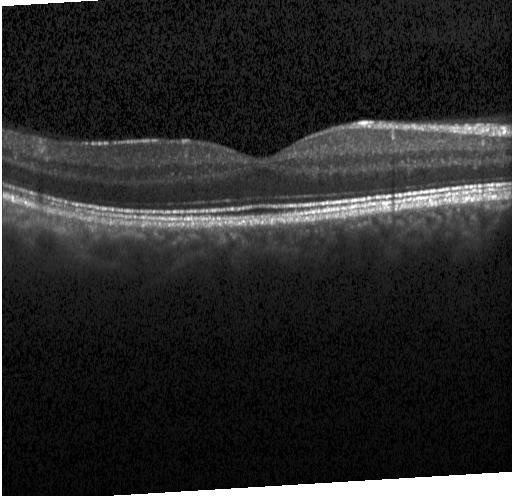 Macular OCT demonstrating no evidence of CNV, DME, or drusen.